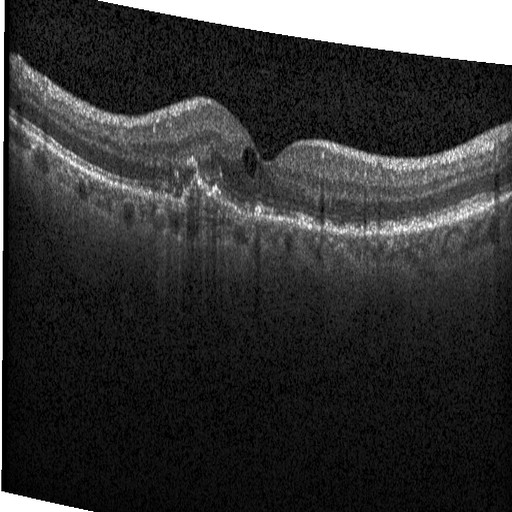 Instrument: Heidelberg Spectralis, horizontal scan through the fovea, OCT B-scan, spectral-domain OCT — Diagnosis: diabetic macular edema (DME).